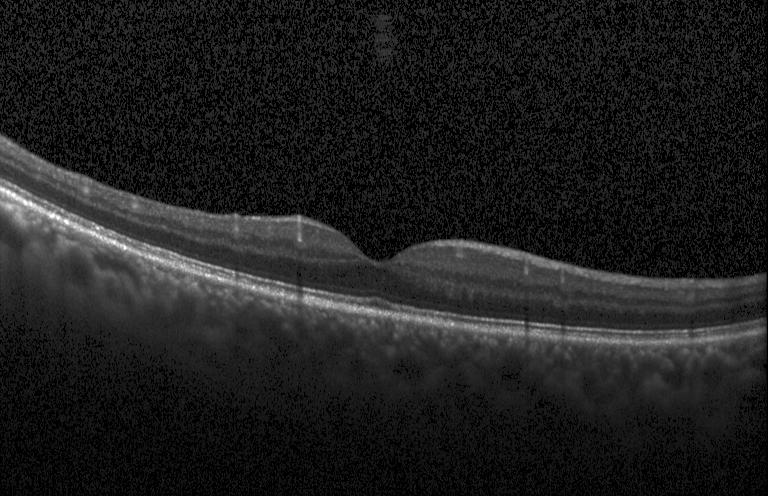
Macular OCT demonstrating neither choroidal neovascularization, diabetic macular edema, nor drusen.